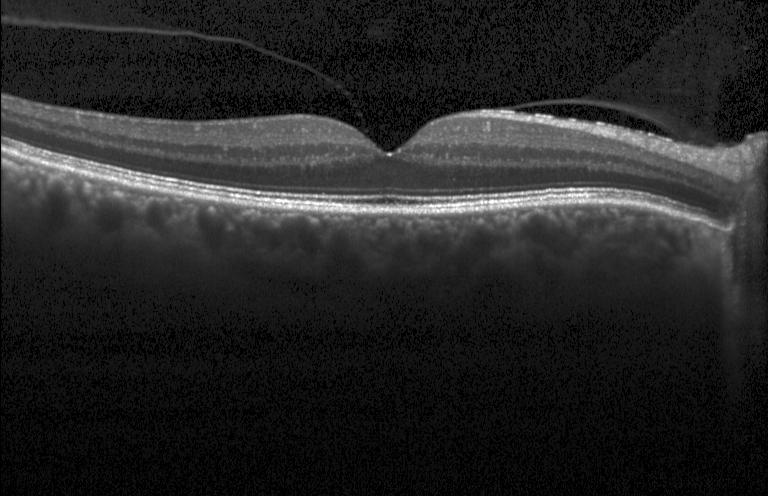 OCT B-scan showing no evidence of CNV, DME, or drusen.